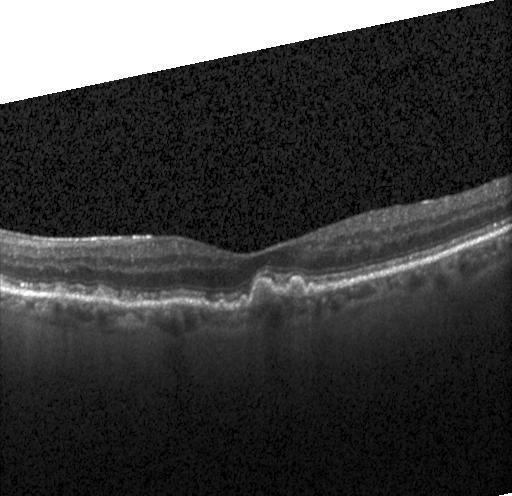 Fovea-centered, instrument: Heidelberg Spectralis, SD-OCT, retinal OCT B-scan.
Assessment: drusen.